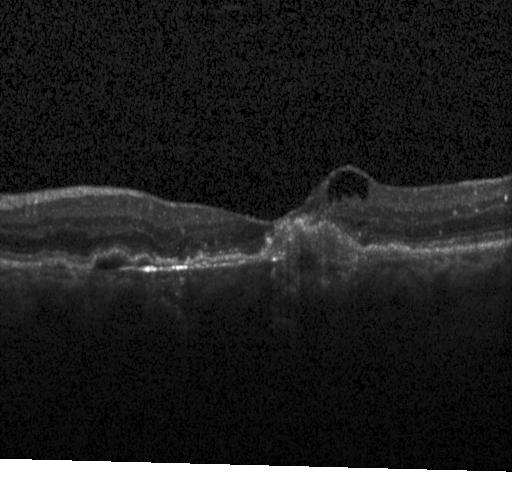 Spectral-domain OCT B-scan: a choroidal neovascular membrane.